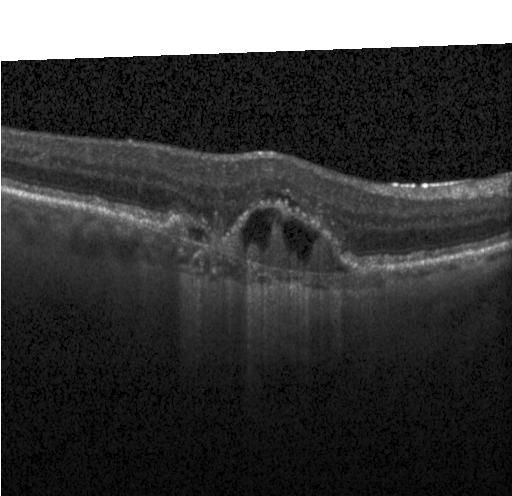 Fovea-centered. OCT B-scan. Diagnosis: a choroidal neovascular membrane.